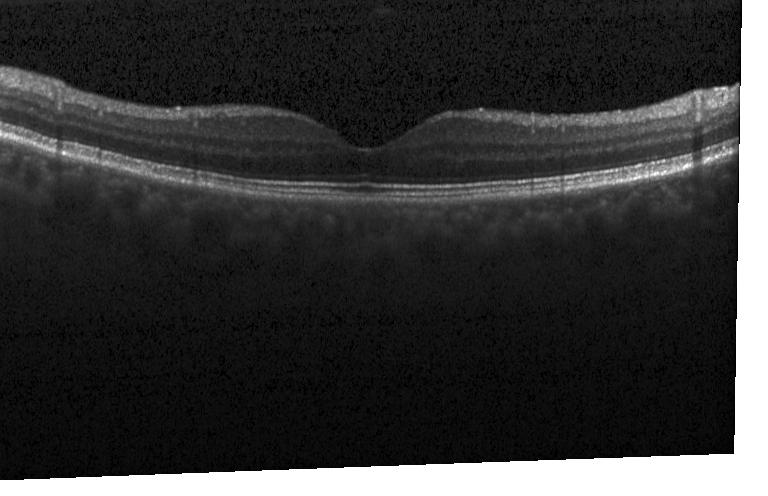

Horizontal scan through the fovea · retinal OCT B-scan — Macular OCT: no choroidal neovascularization, no diabetic macular edema, and no drusen.